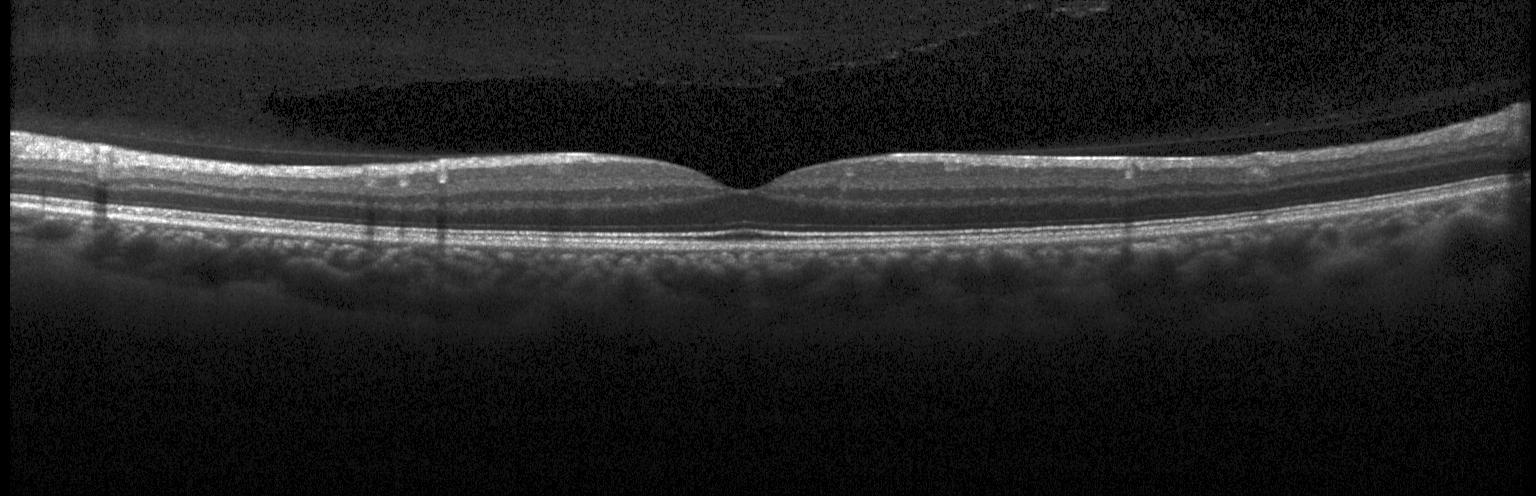
OCT B-scan. Heidelberg Spectralis OCT system. Spectral-domain optical coherence tomography. Macular scan.
Assessment: no choroidal neovascularization, no diabetic macular edema, and no drusen.